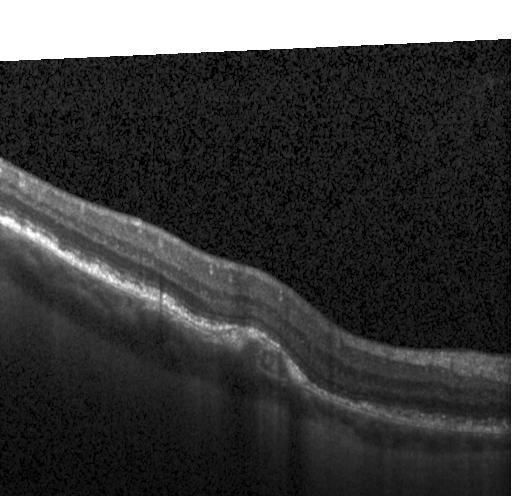
Retinal OCT cross-section; macular scan
Impression: choroidal neovascularization (CNV).